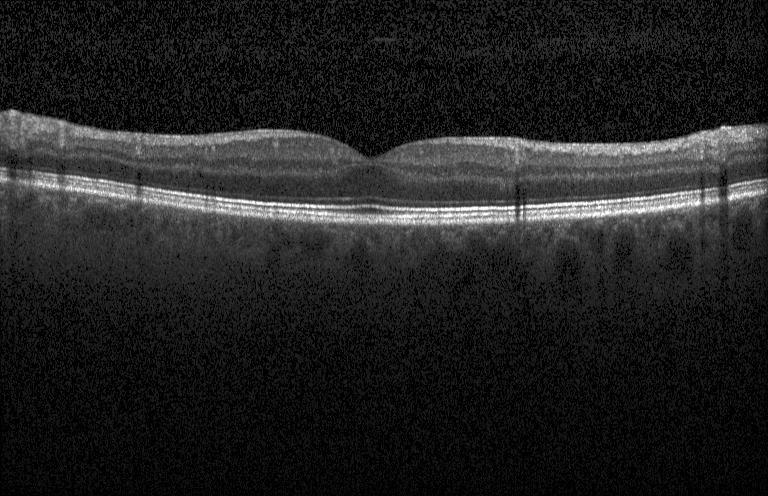 Horizontal scan through the fovea. SD-OCT. Optical coherence tomography scan.
Diagnosis: no choroidal neovascularization, diabetic macular edema, or drusen.